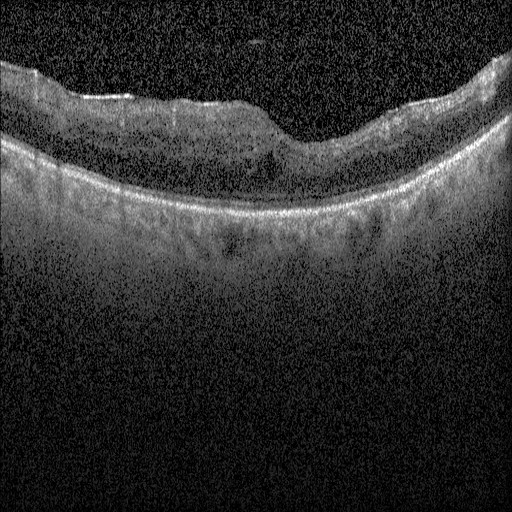

Finding: diabetic macular edema (DME).